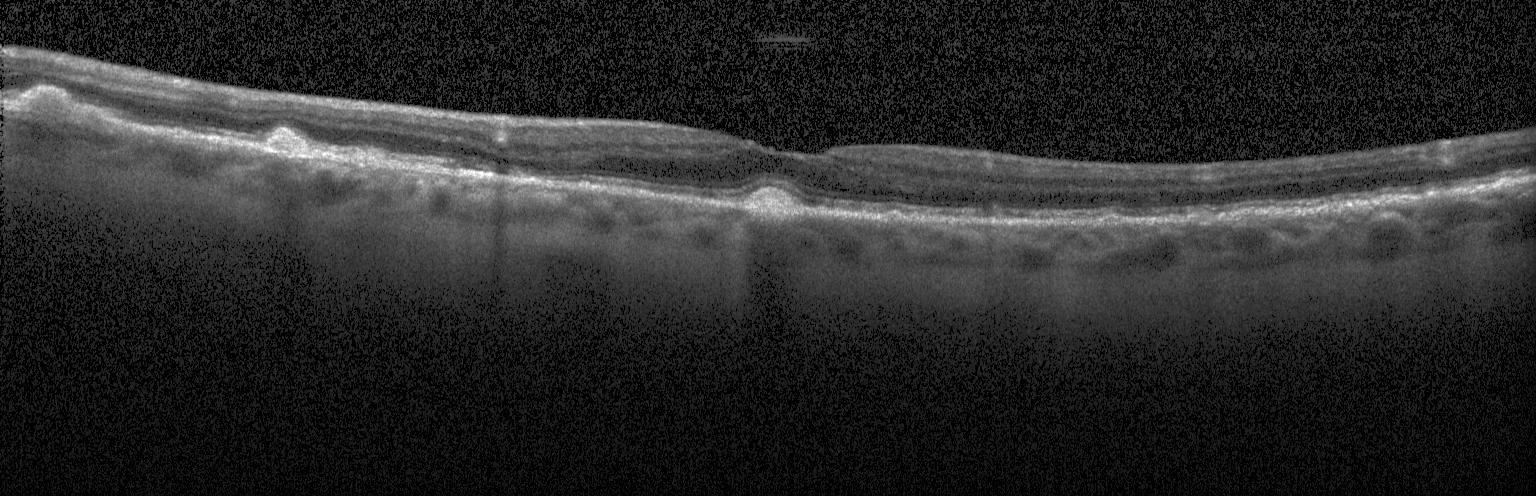
Optical coherence tomography scan · SD-OCT · macular scan · instrument: Heidelberg Spectralis — Finding: multiple drusen.